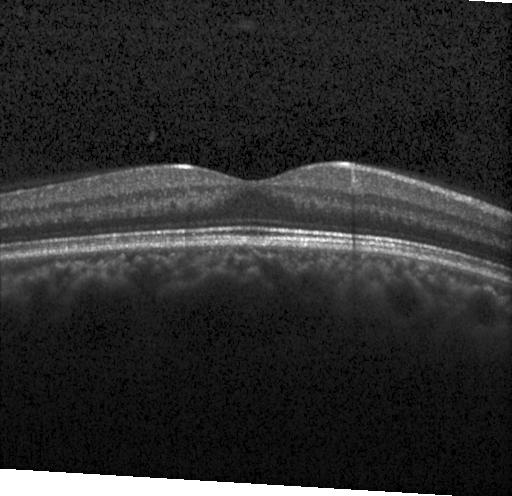

Macular OCT: neither choroidal neovascularization, diabetic macular edema, nor drusen.